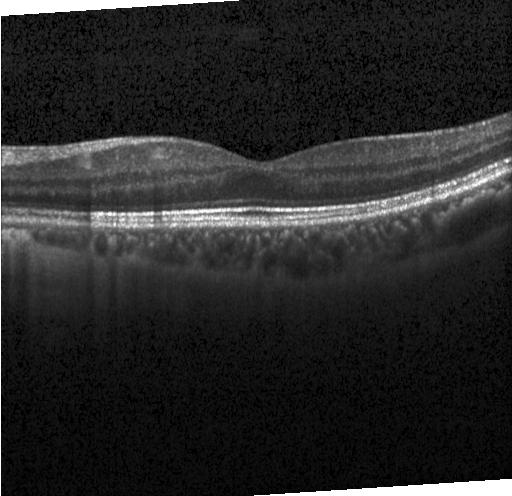
OCT finding: no choroidal neovascularization, diabetic macular edema, or drusen.